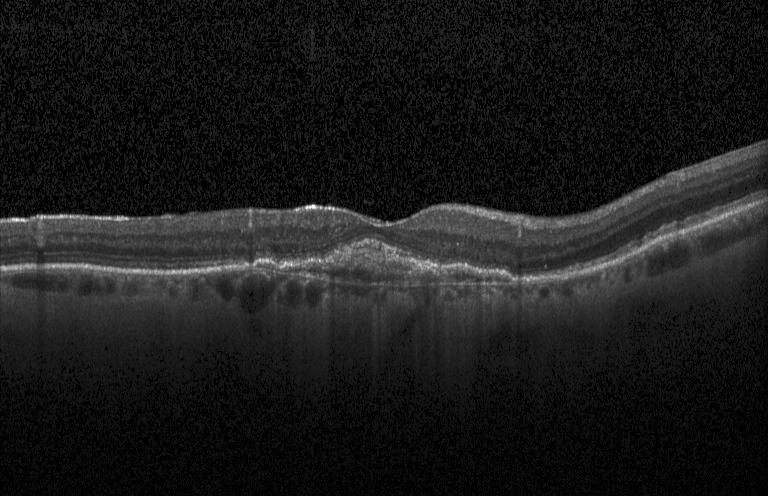 OCT finding: a choroidal neovascular membrane.